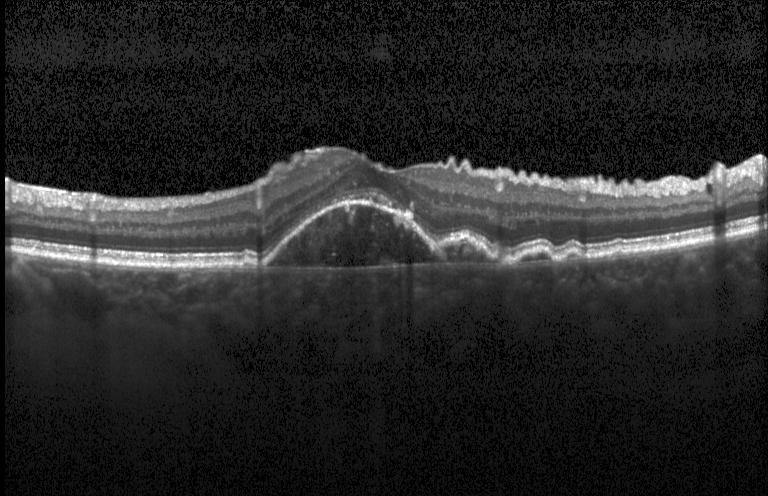
Finding: CNV.